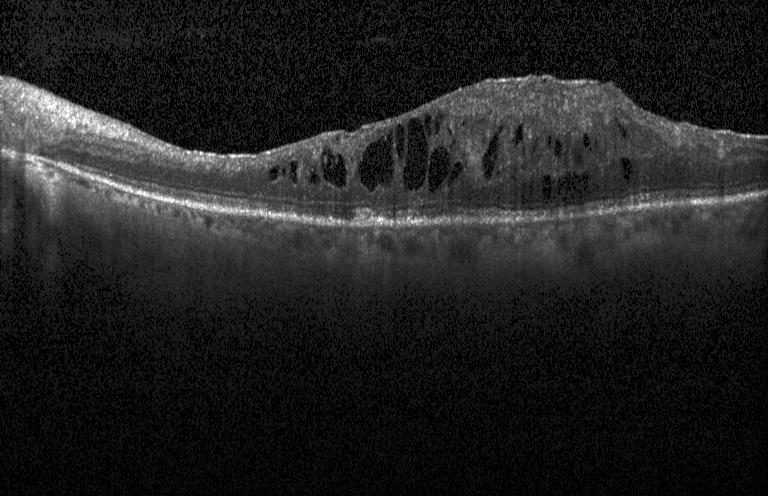
Retinal OCT B-scan — Diagnosis: diabetic macular edema.